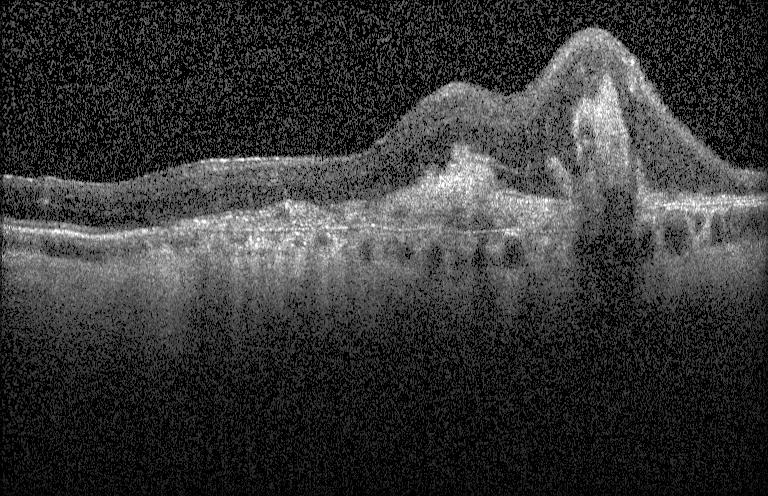
Dx: choroidal neovascularization.